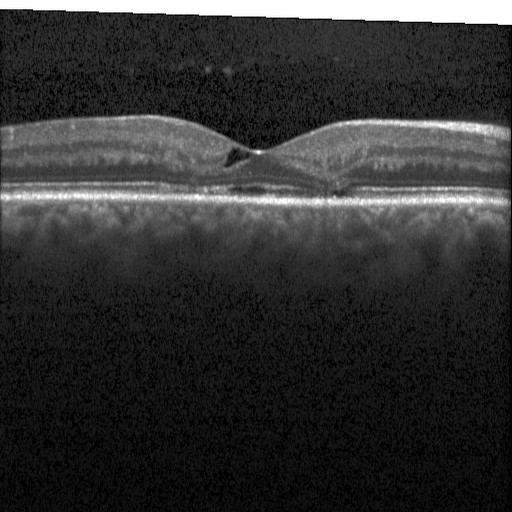

Diagnosis: diabetic macular edema (DME).